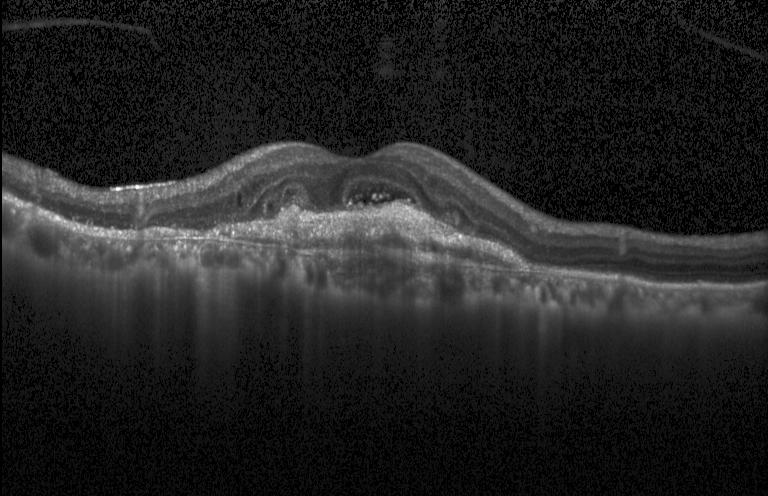

Diagnosis: a choroidal neovascular membrane.